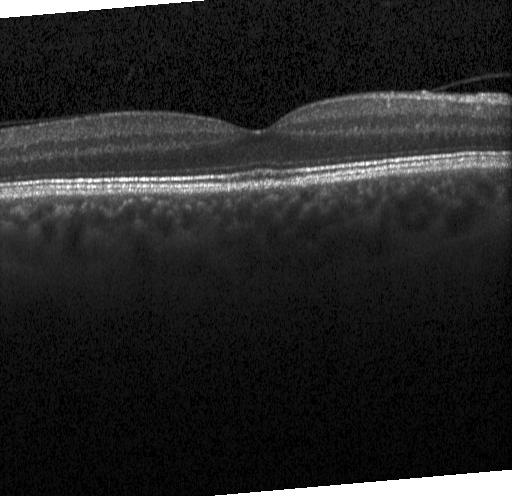
Macular OCT demonstrating no choroidal neovascularization, diabetic macular edema, or drusen.